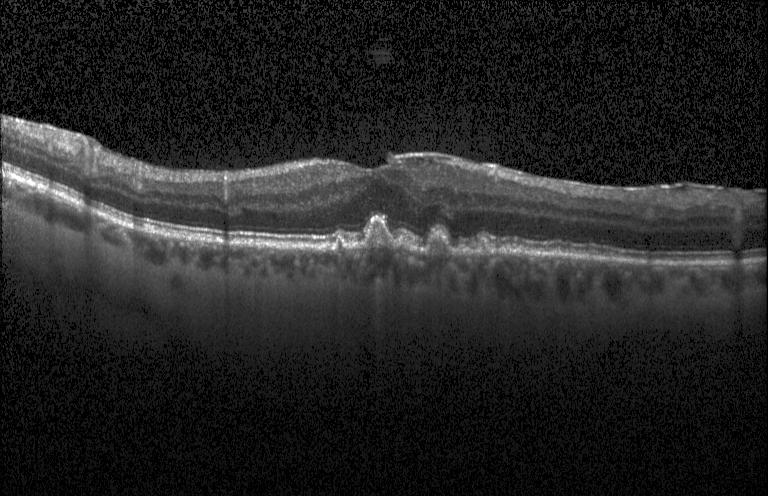

Optical coherence tomography scan. Heidelberg Spectralis OCT system. Through the macula. Spectral-domain optical coherence tomography
Finding: sub-RPE drusenoid deposits.